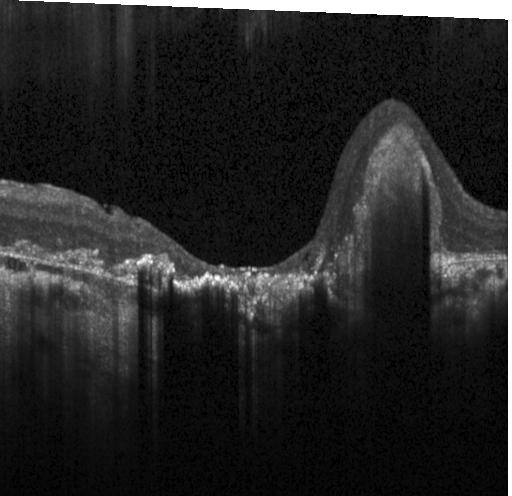
Finding: a choroidal neovascular membrane.